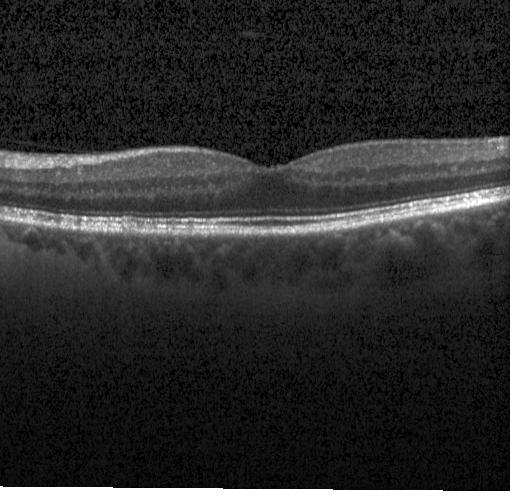
OCT B-scan
Impression: no choroidal neovascularization, diabetic macular edema, or drusen.